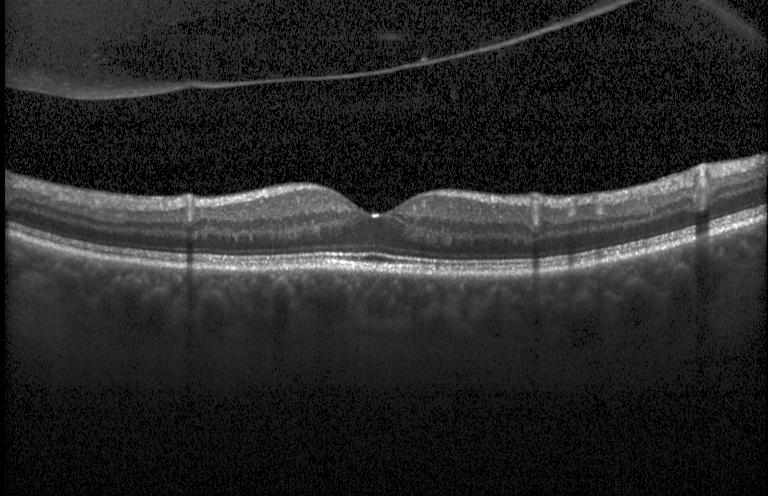

SD-OCT; optical coherence tomography scan; horizontal scan through the fovea; Heidelberg Spectralis OCT system — The scan shows no evidence of choroidal neovascularization, diabetic macular edema, or drusen.